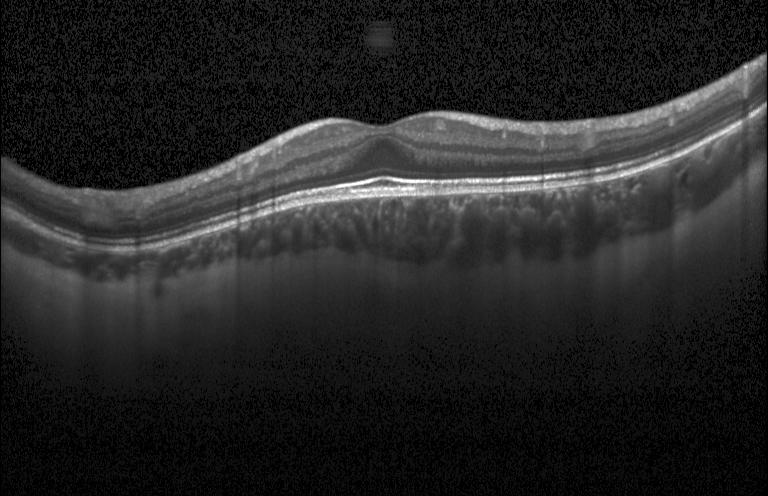
Diagnosis: no choroidal neovascularization, no diabetic macular edema, and no drusen.